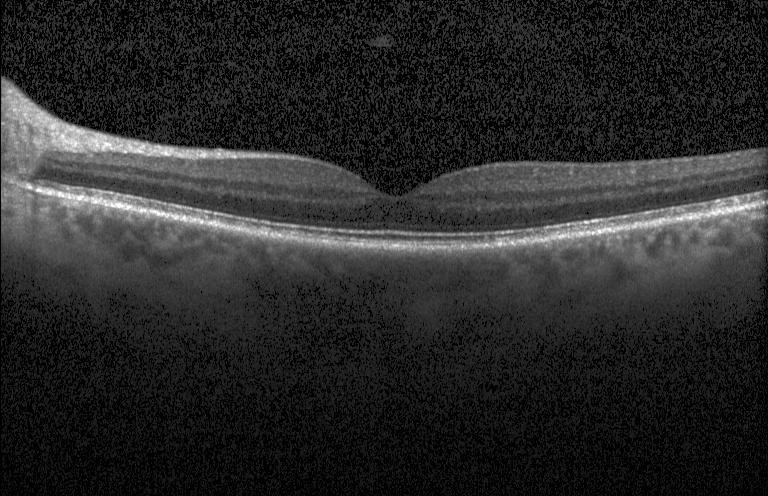

SD-OCT · optical coherence tomography B-scan · fovea-centered
OCT finding: no choroidal neovascularization, diabetic macular edema, or drusen.